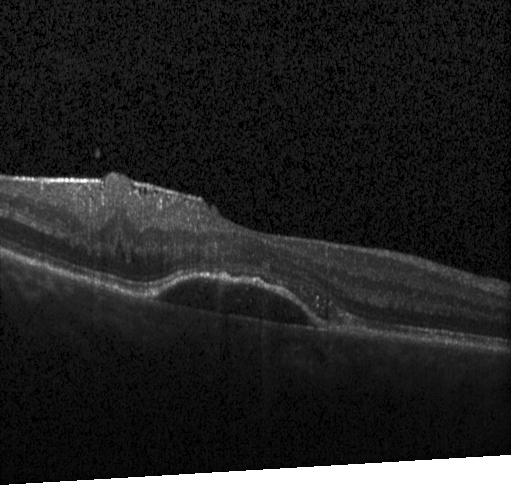

SD-OCT · optical coherence tomography scan
This B-scan demonstrates a choroidal neovascular membrane.